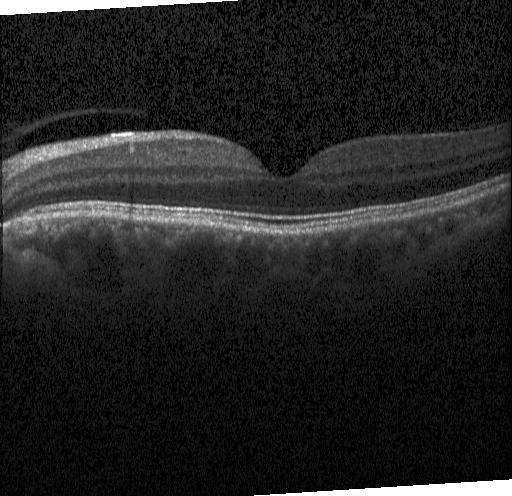 Impression: no evidence of choroidal neovascularization, diabetic macular edema, or drusen.